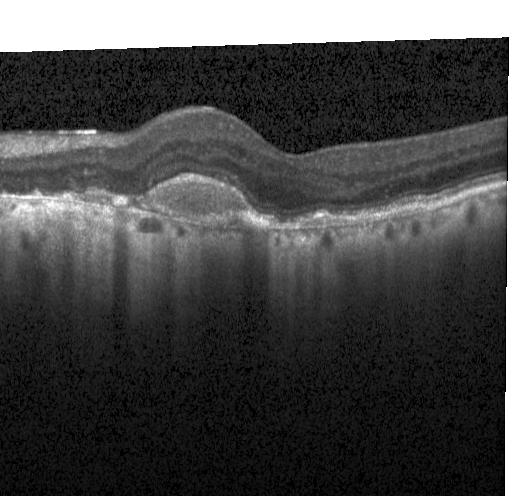 OCT line scan. Spectral-domain optical coherence tomography. Heidelberg Spectralis — Assessment: choroidal neovascularization (CNV).